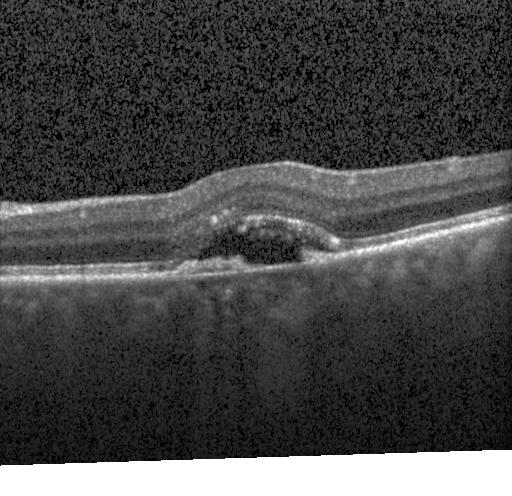
Diagnosis: a choroidal neovascular membrane.